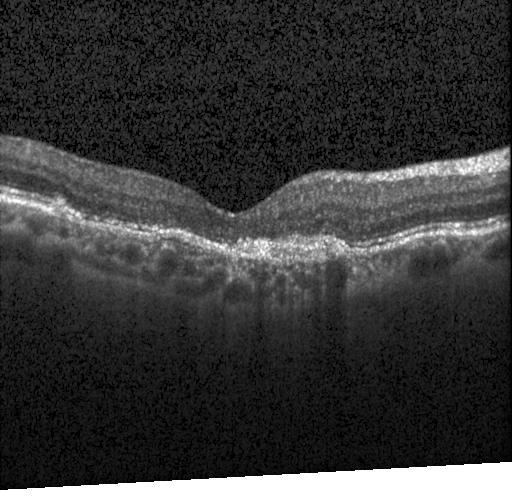
CNV.